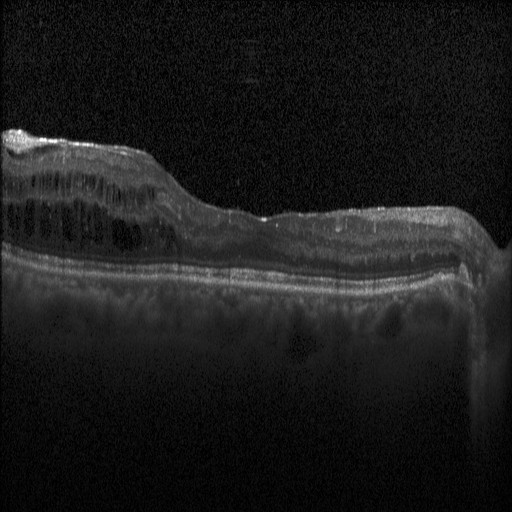

Heidelberg Spectralis · retinal OCT cross-section. Finding: diabetic macular edema.